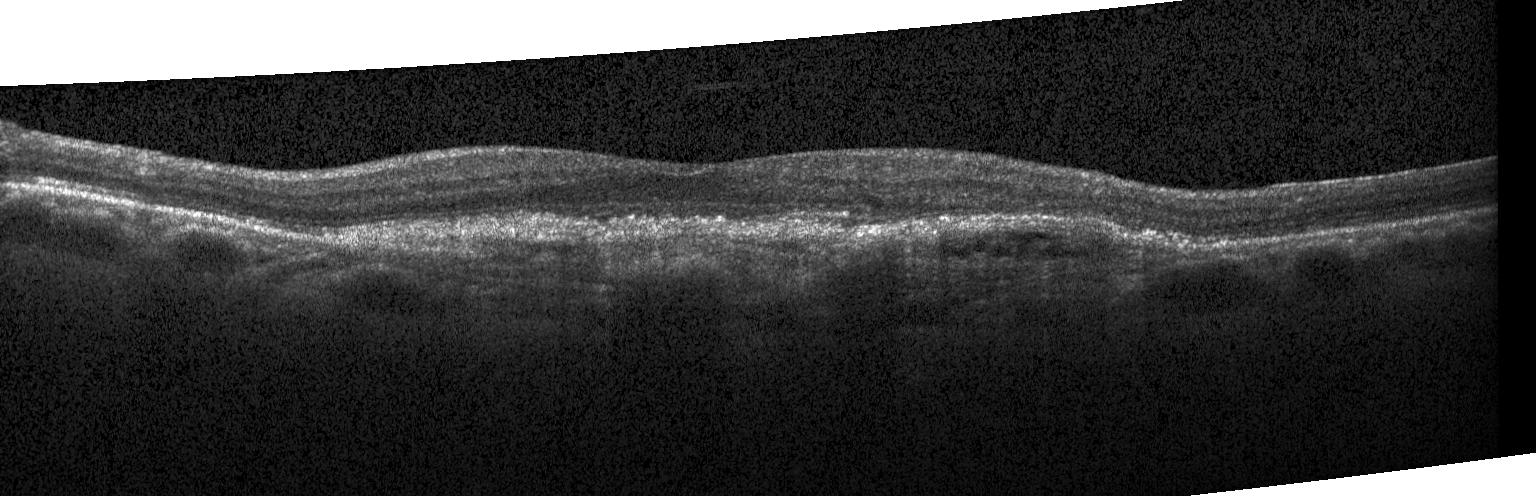

Retinal OCT cross-section
Finding: choroidal neovascularization (CNV).